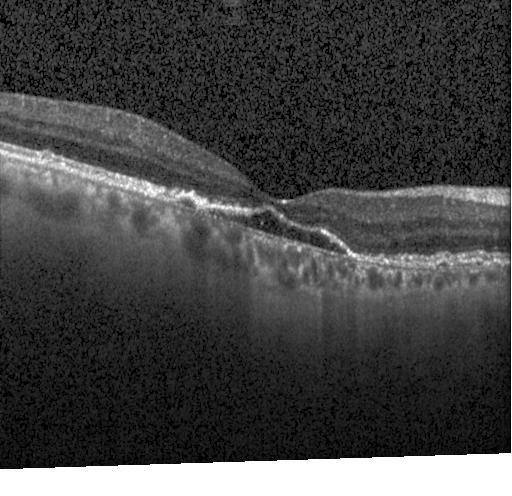 Finding: choroidal neovascularization.